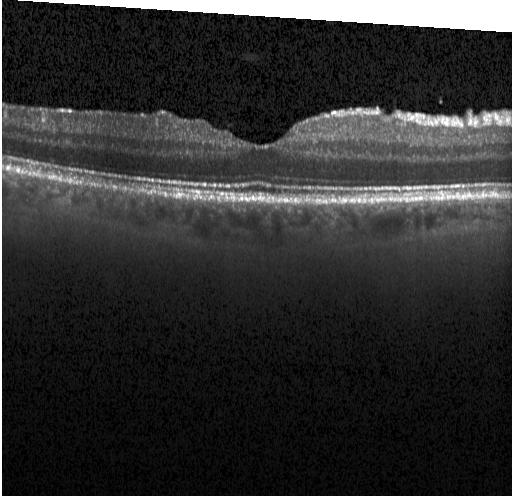 Fovea-centered, OCT B-scan, instrument: Heidelberg Spectralis, SD-OCT. This B-scan demonstrates neither choroidal neovascularization, diabetic macular edema, nor drusen.